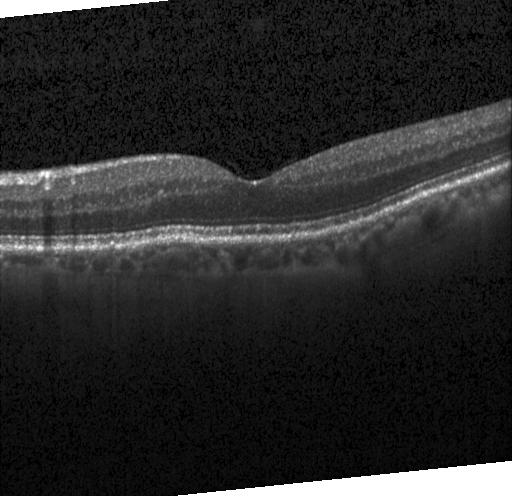
Retinal OCT cross-section · centered on the fovea — OCT finding: no choroidal neovascularization, diabetic macular edema, or drusen.